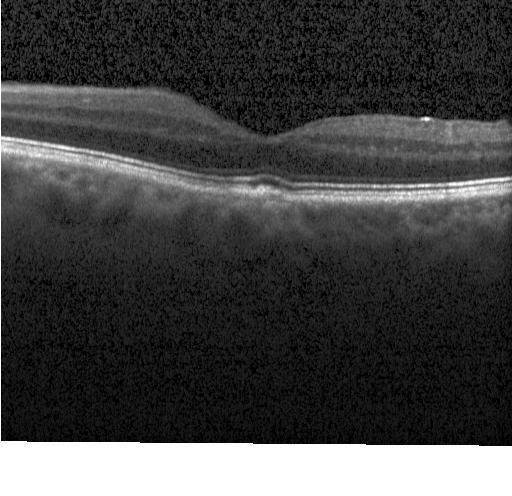 Macular OCT: drusen.